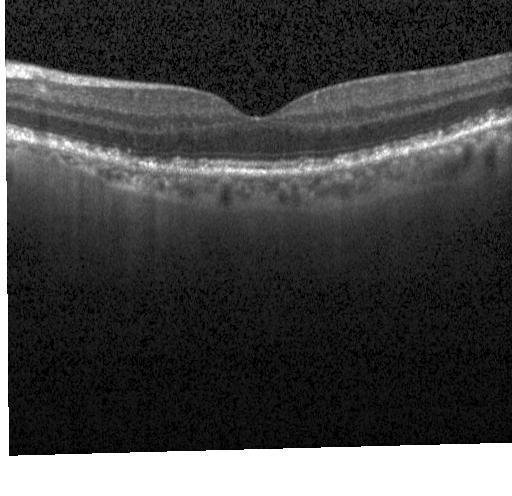
Spectral-domain OCT B-scan: sub-RPE drusenoid deposits.